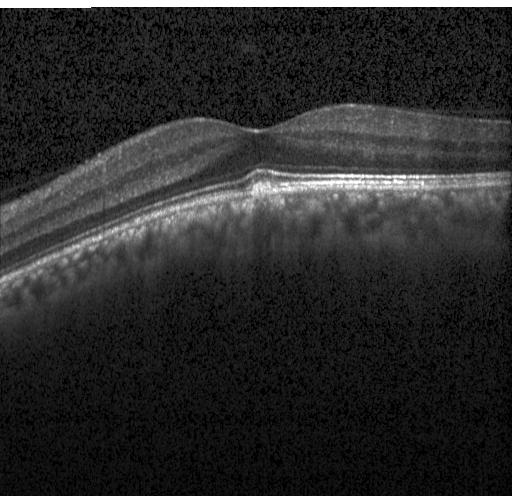 Spectral-domain OCT; retinal OCT B-scan; horizontal scan through the fovea. Diagnosis: no choroidal neovascularization, diabetic macular edema, or drusen.